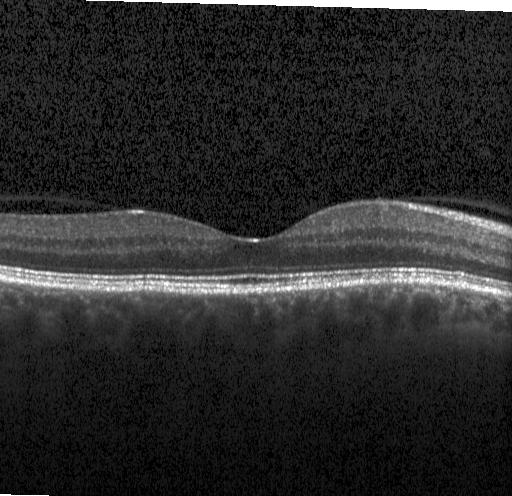 The scan shows no evidence of choroidal neovascularization, diabetic macular edema, or drusen.